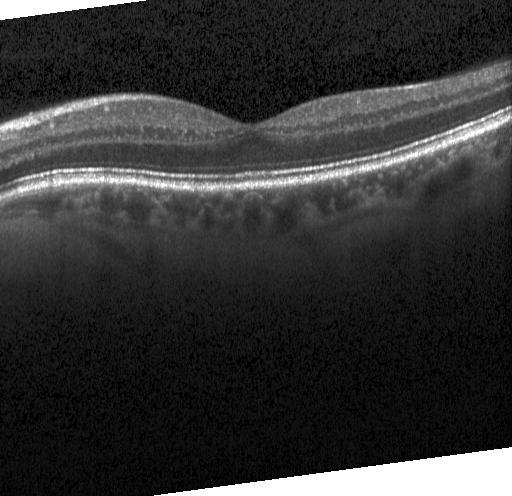
Dx: no CNV, no DME, and no drusen.